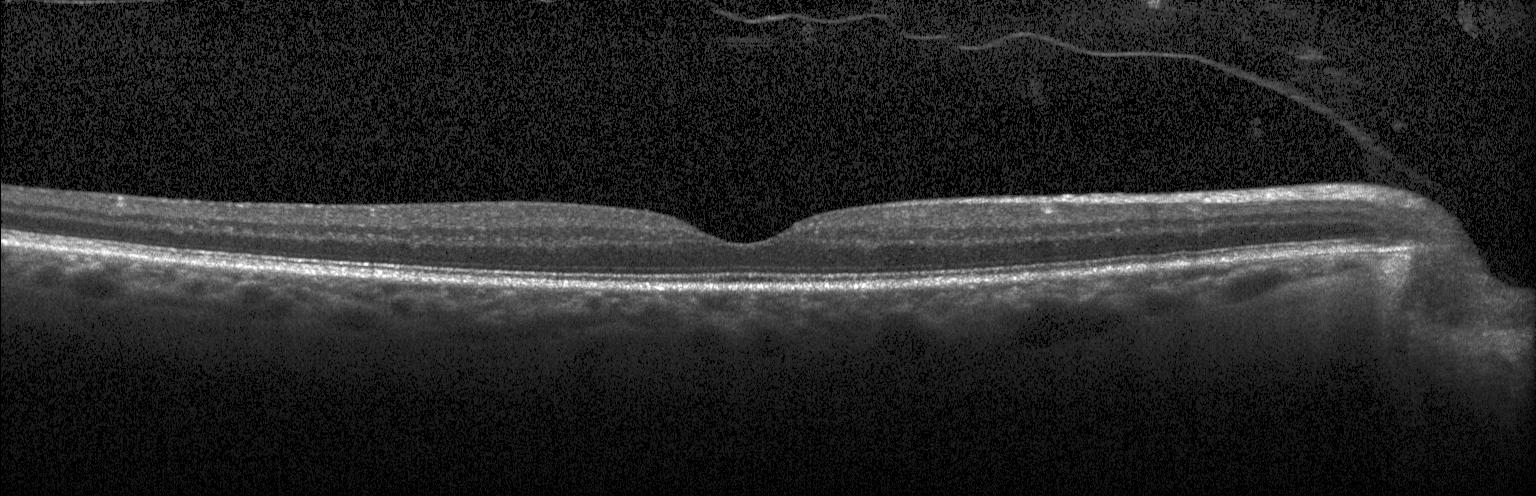

Optical coherence tomography B-scan. Diagnosis: no CNV, no DME, and no drusen.